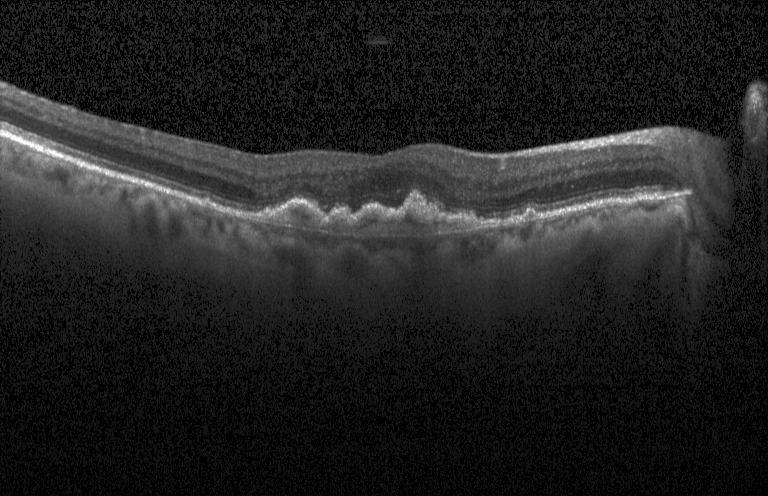
Macular scan. Spectral-domain optical coherence tomography. Optical coherence tomography scan. Acquired on a Heidelberg Spectralis
Finding: choroidal neovascularization.